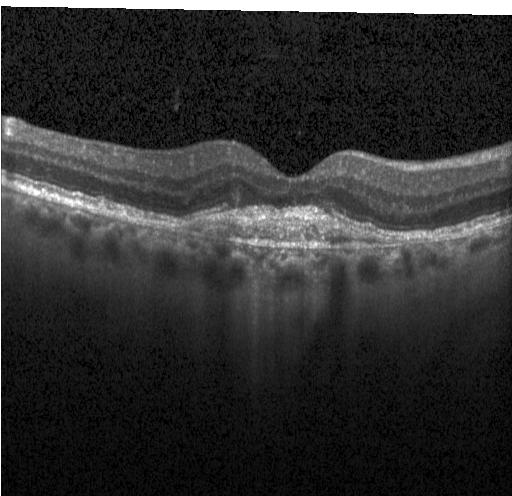
Macular OCT demonstrating a choroidal neovascular membrane.